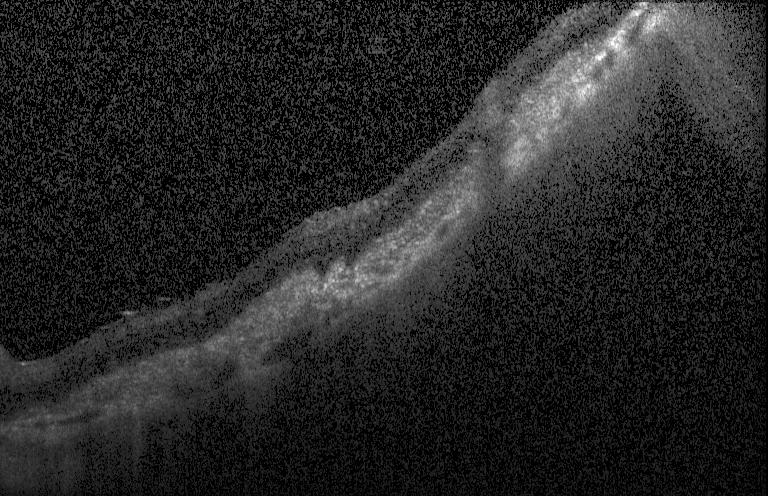

OCT B-scan. The scan shows a choroidal neovascular membrane.